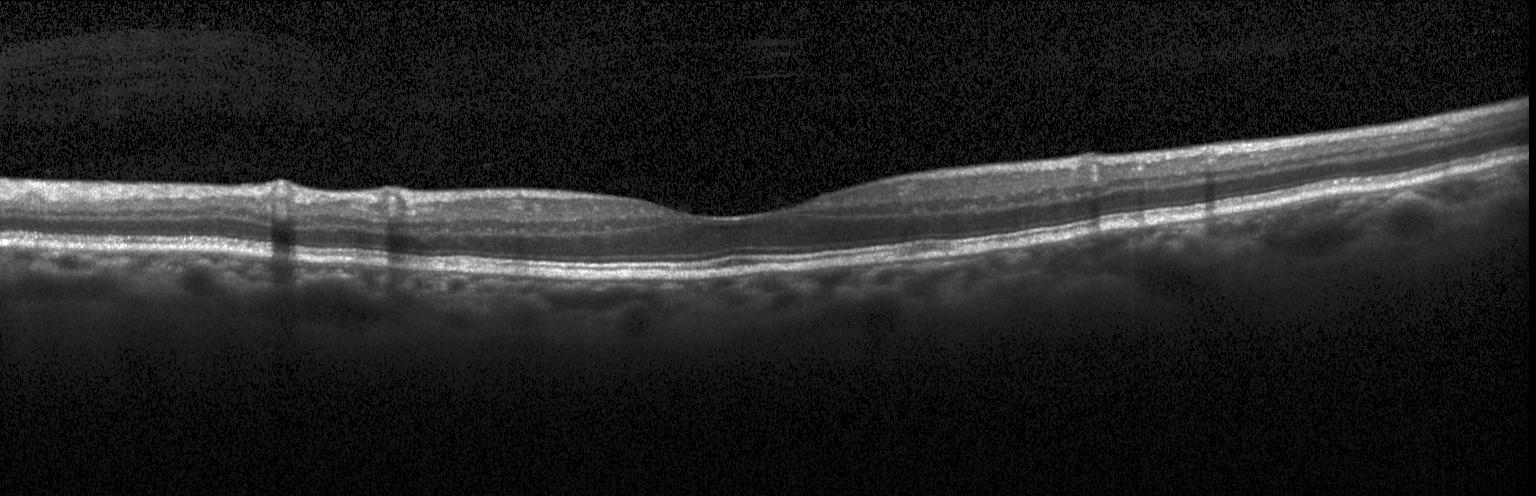

OCT finding: no evidence of choroidal neovascularization, diabetic macular edema, or drusen.